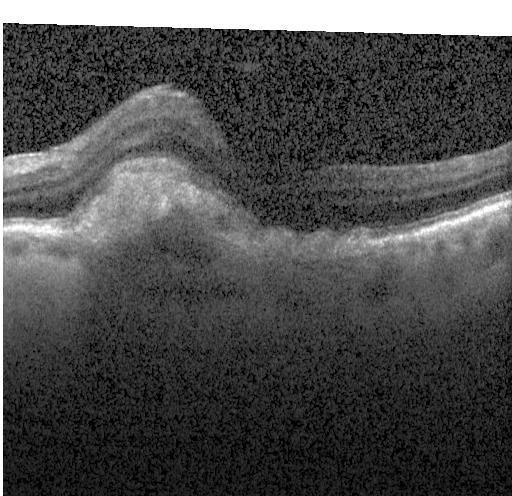
Assessment: choroidal neovascularization (CNV).